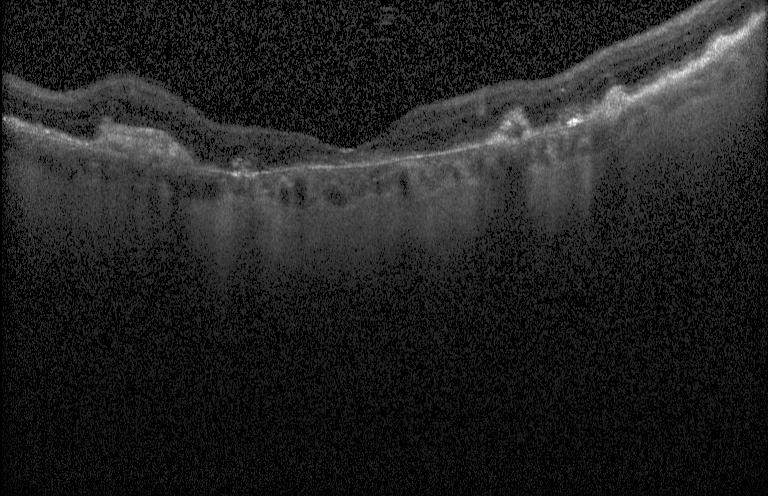

Impression: choroidal neovascularization.